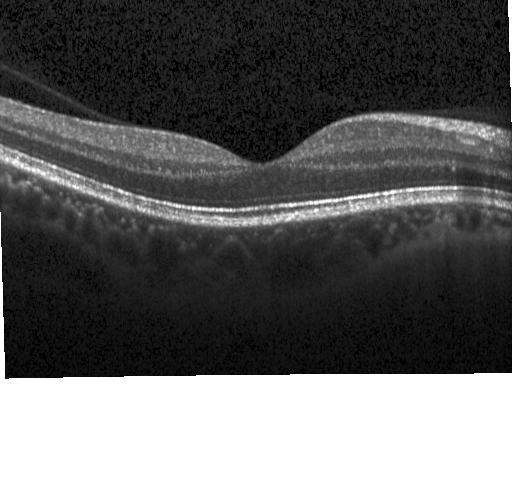
OCT B-scan; SD-OCT
Finding: no choroidal neovascularization, diabetic macular edema, or drusen.